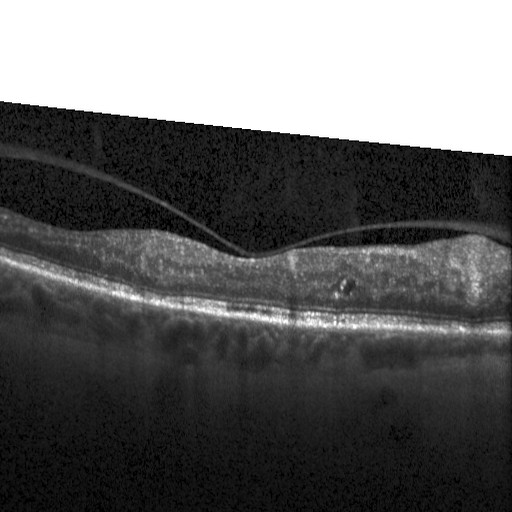 Spectral-domain OCT B-scan: diabetic macular edema (DME).